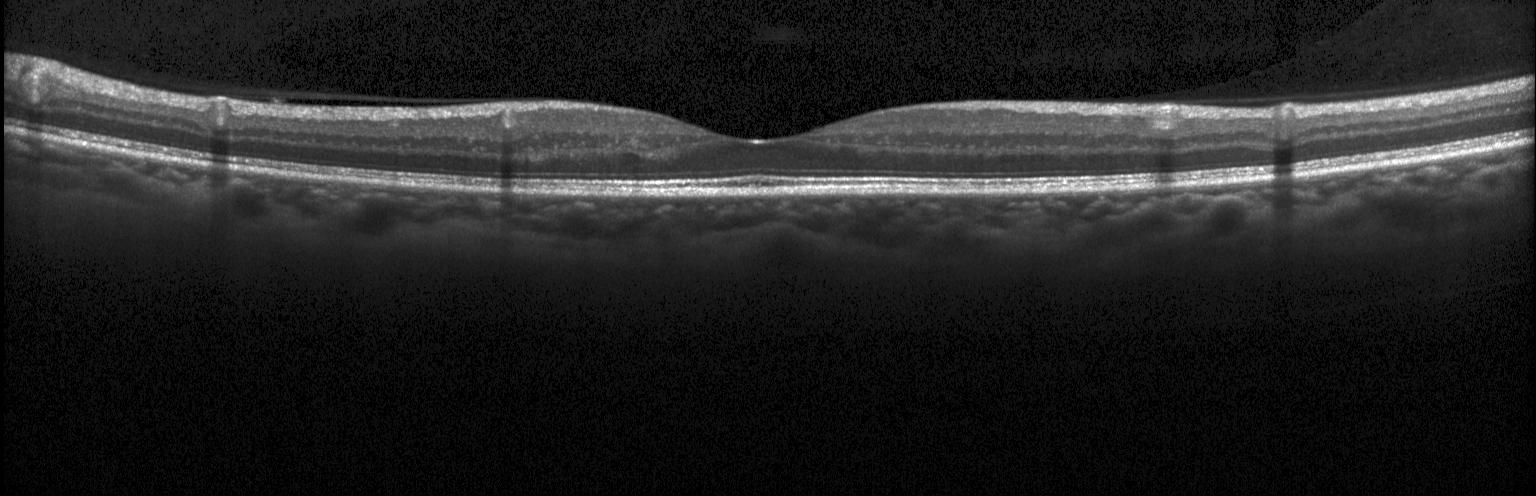
OCT finding: no CNV, no DME, and no drusen.